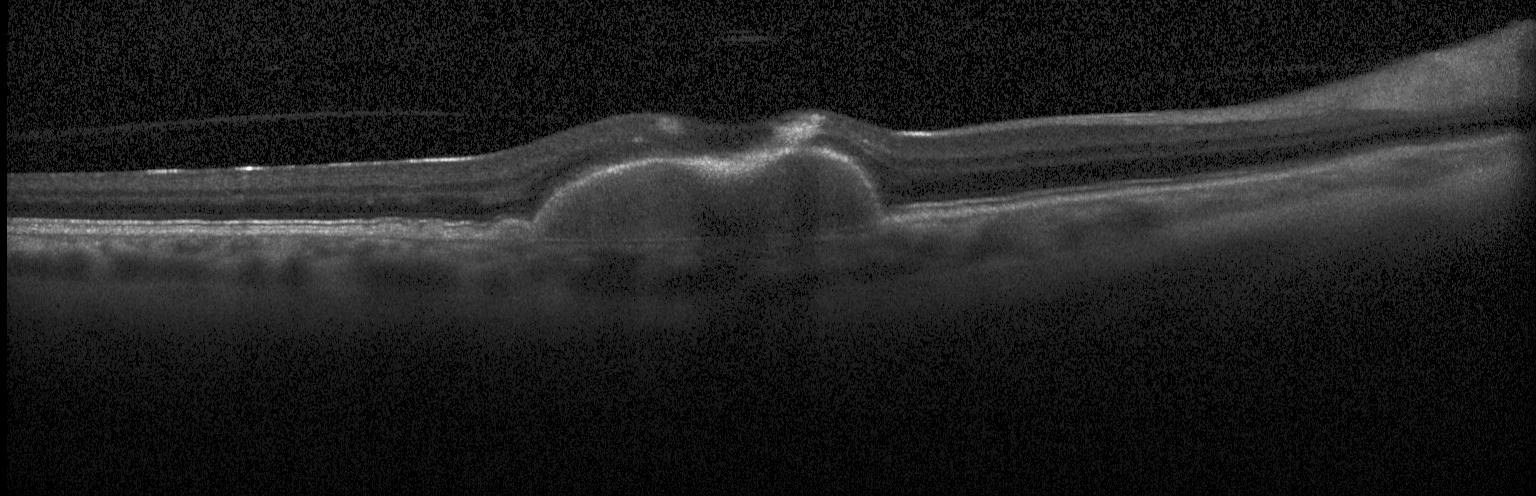
Finding: a choroidal neovascular membrane.